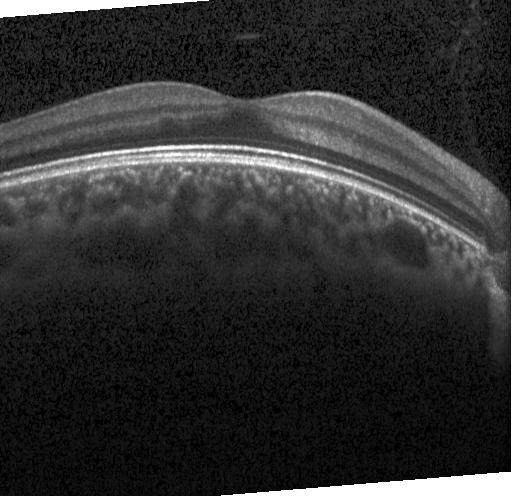
Impression: no choroidal neovascularization, diabetic macular edema, or drusen.